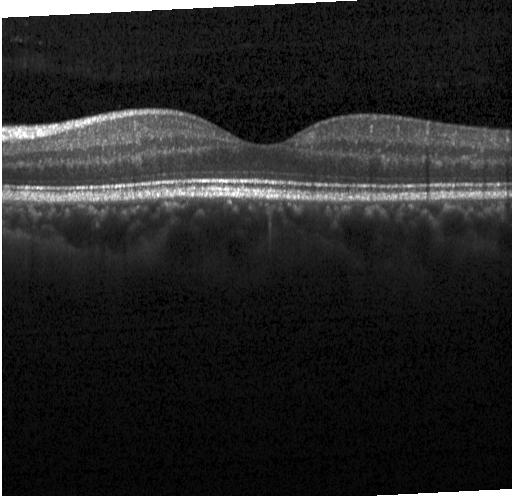
OCT line scan. This B-scan demonstrates no evidence of choroidal neovascularization, diabetic macular edema, or drusen.